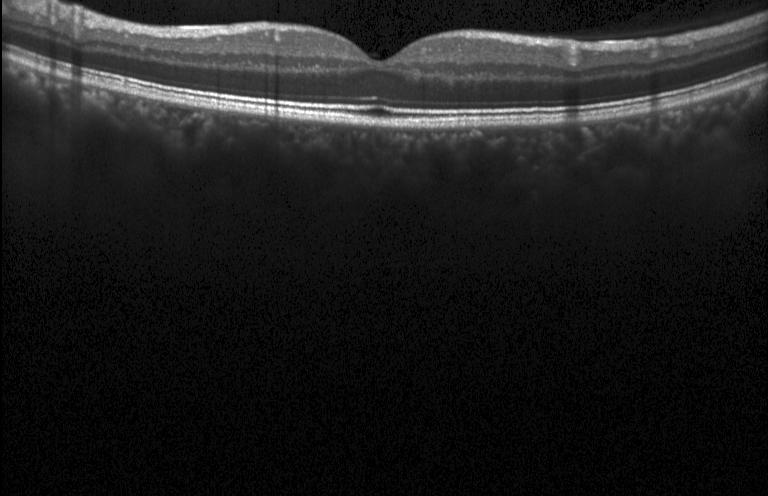
SD-OCT, OCT line scan.
Impression: no CNV, DME, or drusen.